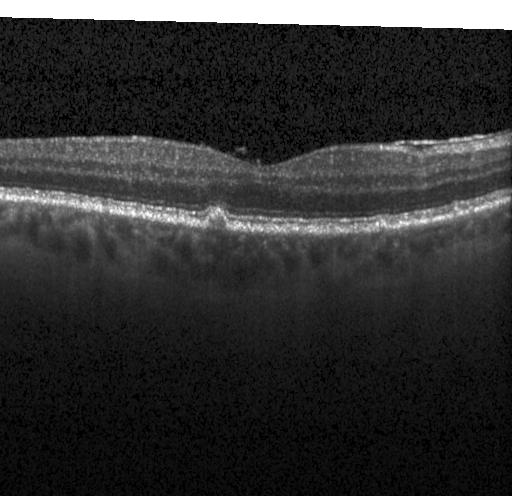 Macular OCT: sub-RPE drusenoid deposits.